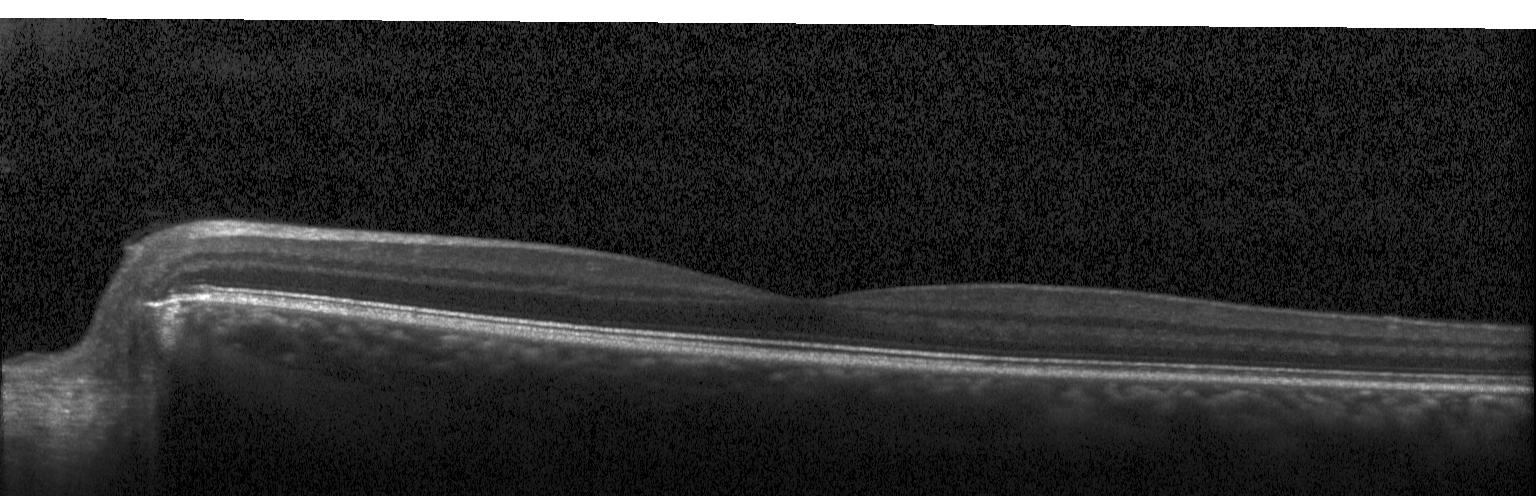
SD-OCT · macular scan · OCT B-scan
OCT finding: no CNV, no DME, and no drusen.